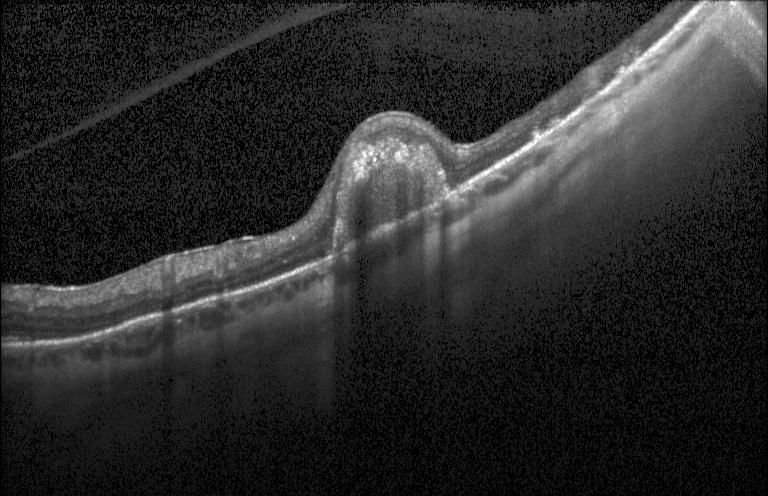 Dx: a choroidal neovascular membrane.